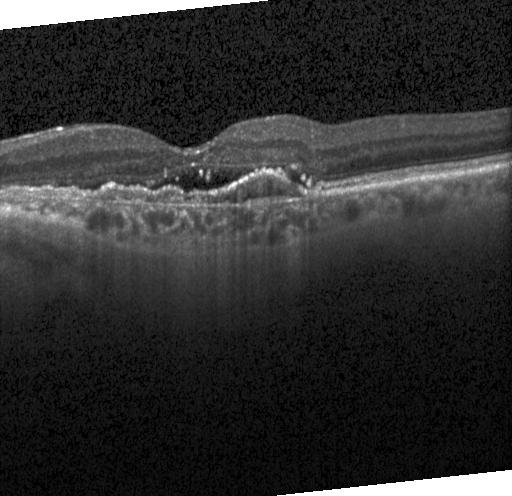 Retinal OCT cross-section showing a choroidal neovascular membrane.